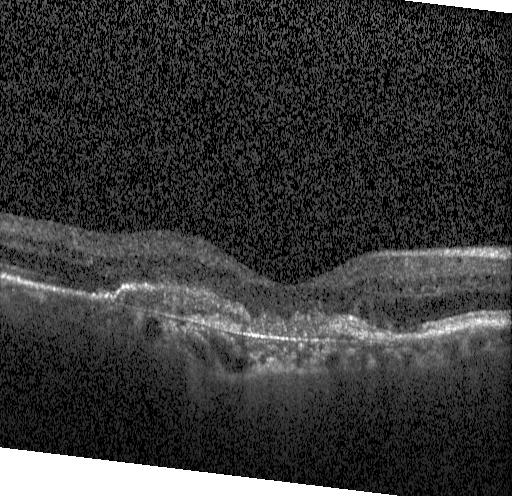
Retinal OCT cross-section. Heidelberg Spectralis OCT system. Centered on the fovea.
Assessment: CNV.